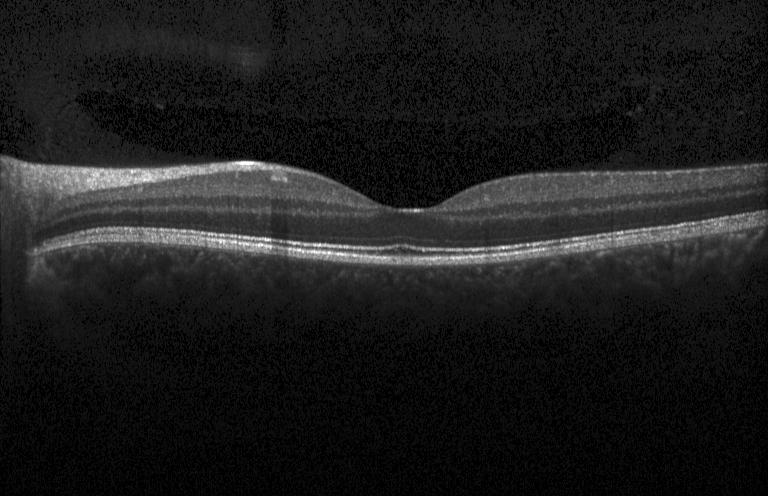 Retinal OCT cross-section — The scan shows no CNV, no DME, and no drusen.